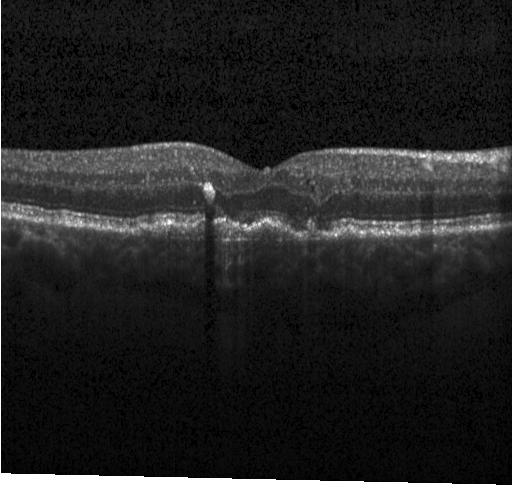
Retinal OCT B-scan; spectral-domain OCT; macular scan; Heidelberg Spectralis. Dx: a choroidal neovascular membrane.